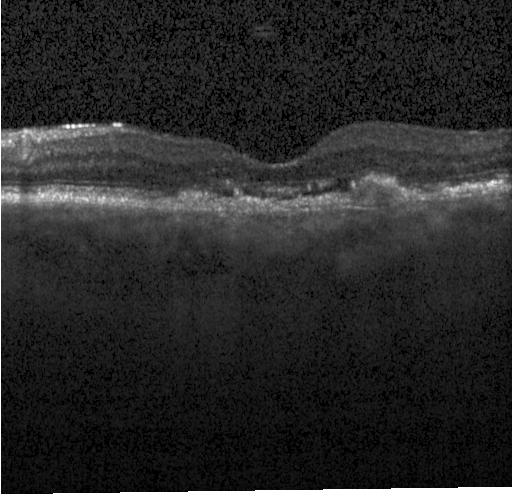

Spectral-domain OCT, Heidelberg Spectralis OCT system, optical coherence tomography scan.
Impression: a choroidal neovascular membrane.